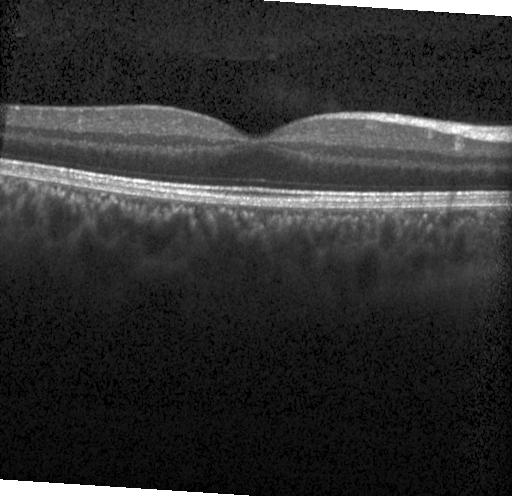
Spectral-domain OCT · OCT B-scan — Impression: no evidence of choroidal neovascularization, diabetic macular edema, or drusen.